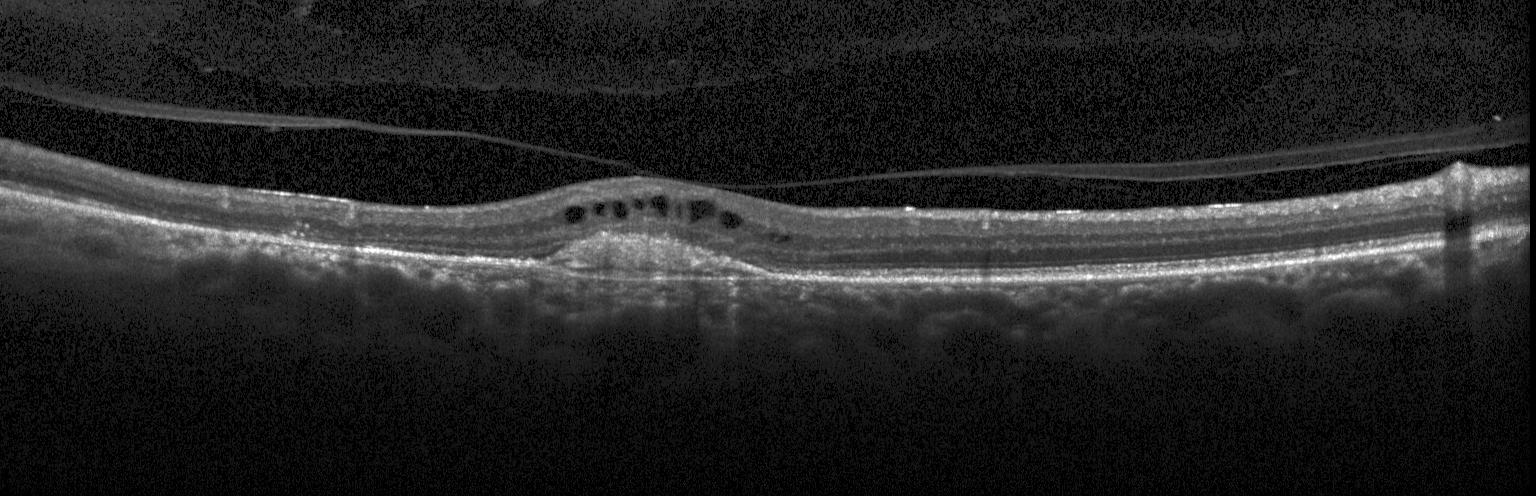

Spectral-domain OCT. Through the macula. Retinal OCT B-scan. Diagnosis: a choroidal neovascular membrane.